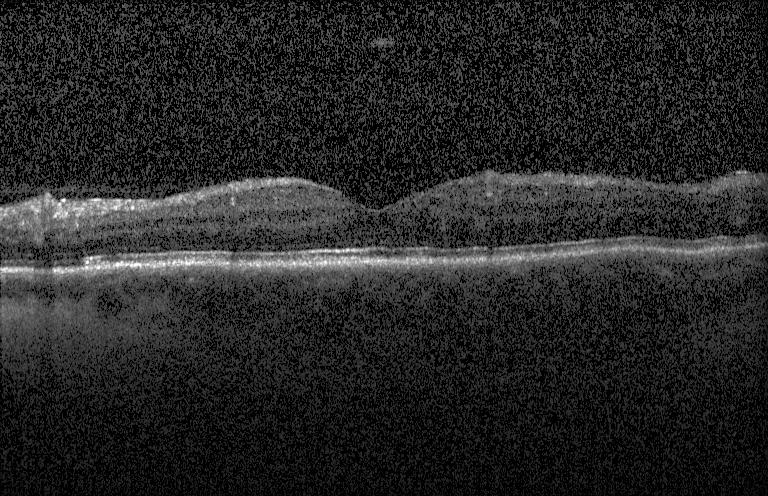

Optical coherence tomography scan. Macular OCT: diabetic macular edema.